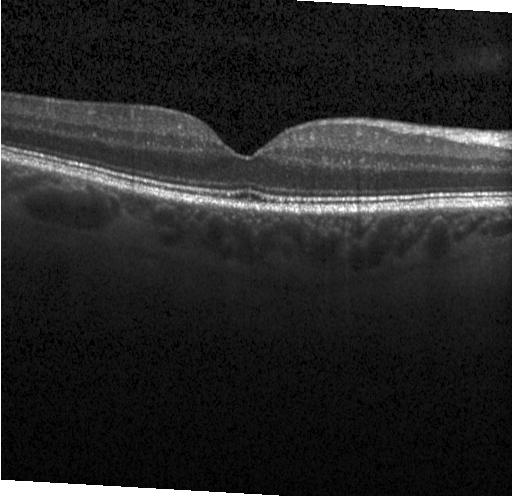
Impression: no evidence of choroidal neovascularization, diabetic macular edema, or drusen.